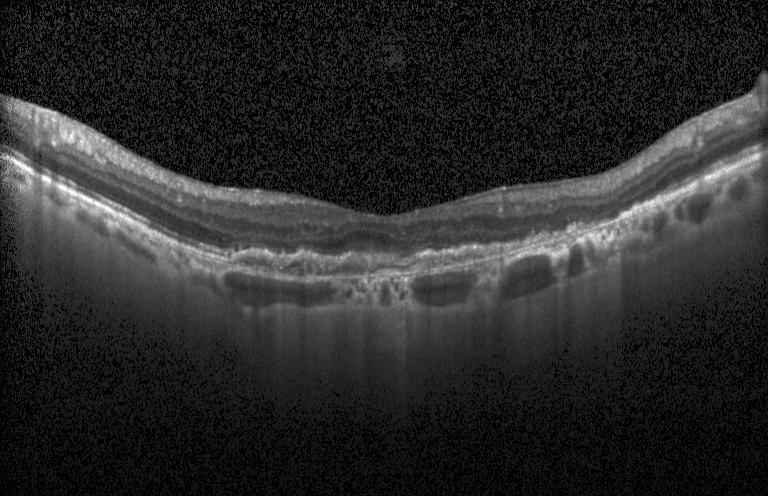

Impression: choroidal neovascularization (CNV).